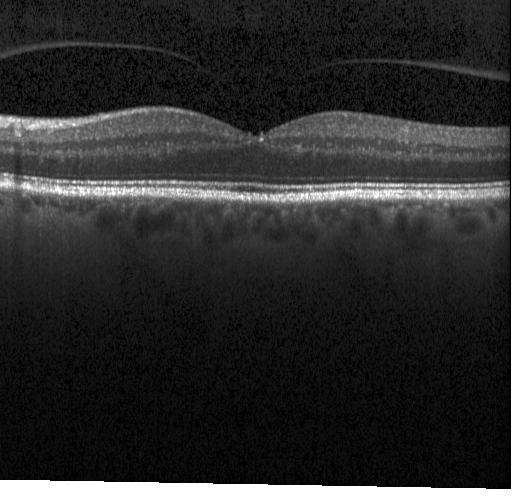

Diagnosis: no evidence of choroidal neovascularization, diabetic macular edema, or drusen.